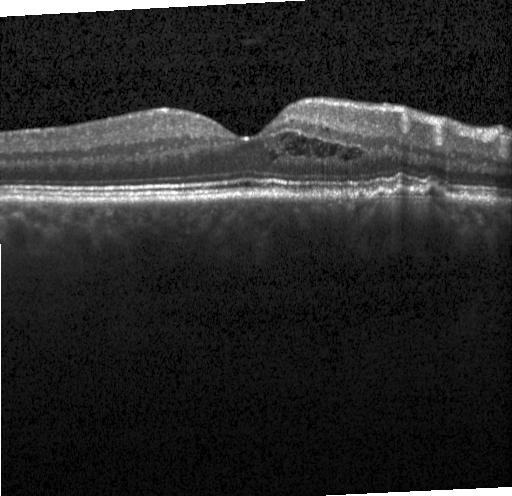
Horizontal scan through the fovea, retinal OCT B-scan, spectral-domain optical coherence tomography, acquired on a Heidelberg Spectralis — This B-scan demonstrates choroidal neovascularization.